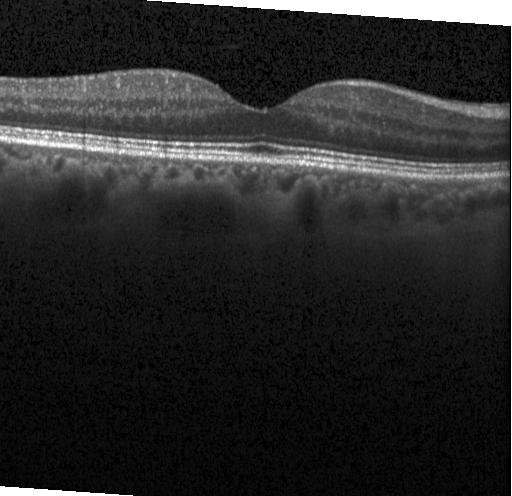

Optical coherence tomography scan. Instrument: Heidelberg Spectralis. The scan shows no choroidal neovascularization, no diabetic macular edema, and no drusen.